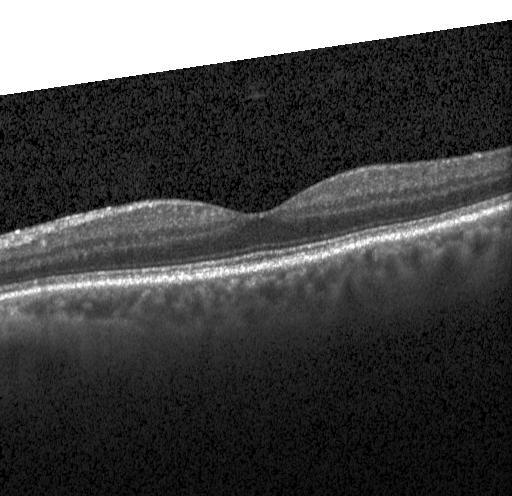

Retinal OCT cross-section
No choroidal neovascularization, no diabetic macular edema, and no drusen.